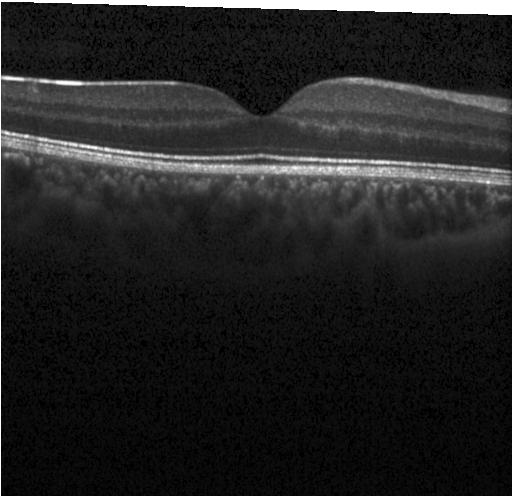 Finding: no choroidal neovascularization, diabetic macular edema, or drusen.